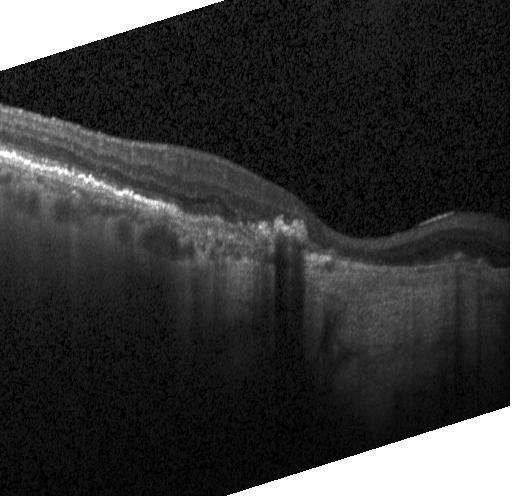
Retinal OCT B-scan. Diagnosis: a choroidal neovascular membrane.